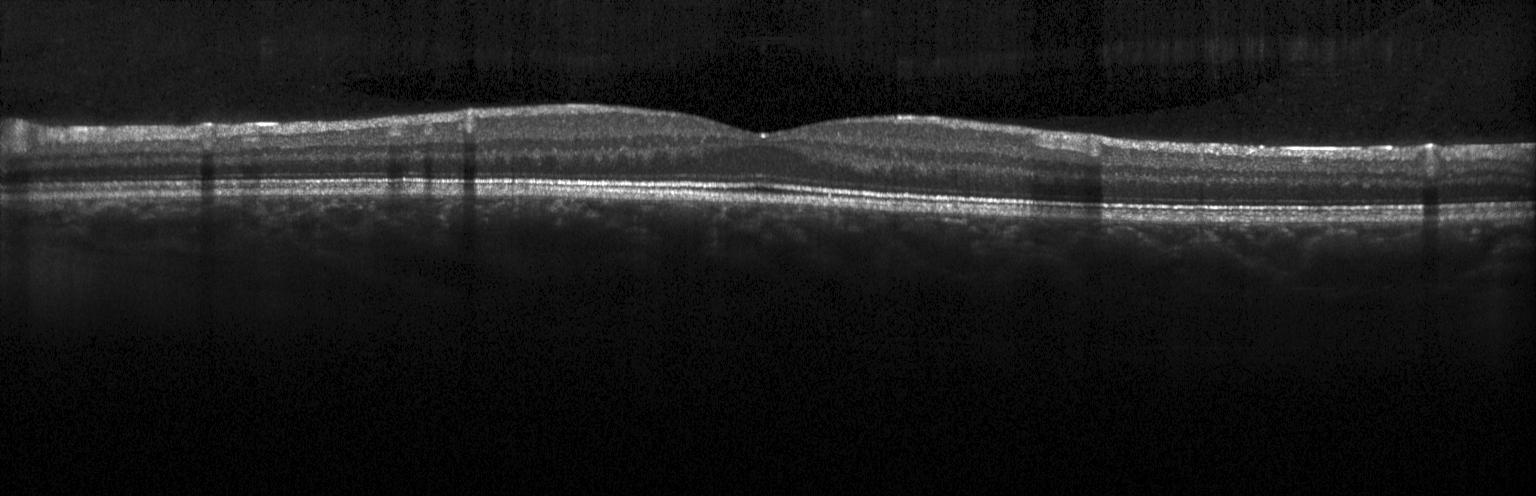
OCT line scan — Macular OCT: neither choroidal neovascularization, diabetic macular edema, nor drusen.